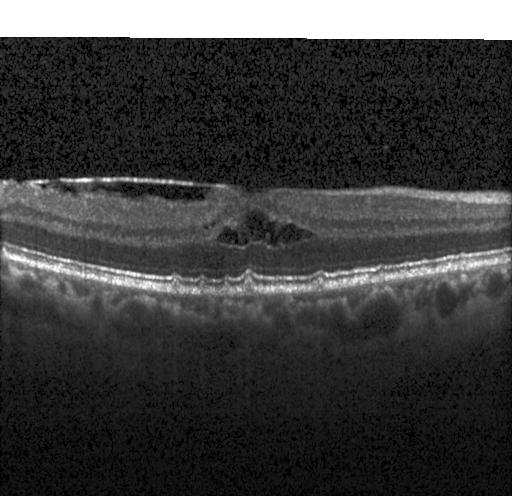 Finding: drusen.